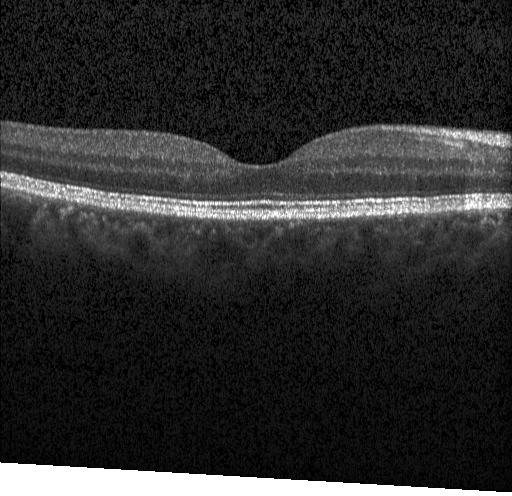
Dx: no evidence of CNV, DME, or drusen.